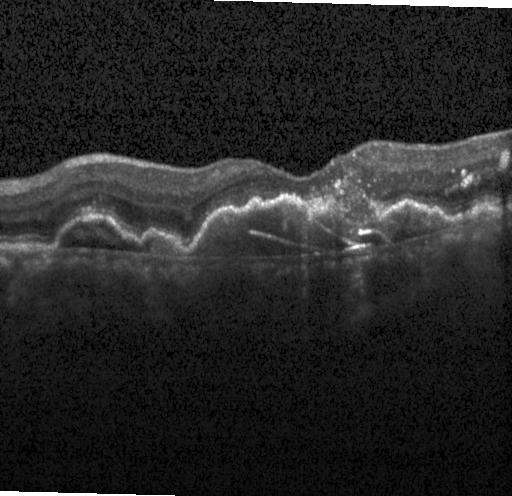

OCT B-scan. Dx: a choroidal neovascular membrane.